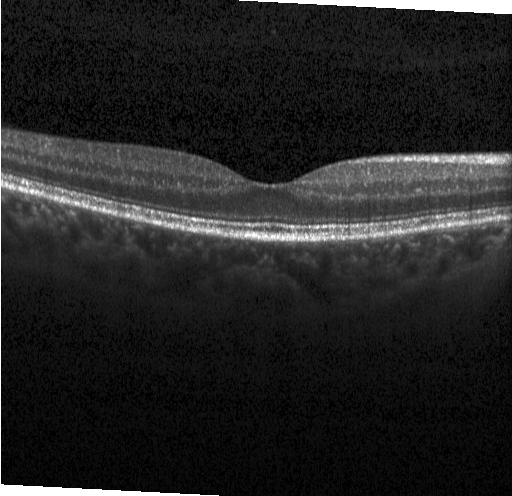 Spectral-domain optical coherence tomography · OCT line scan — Assessment: no evidence of choroidal neovascularization, diabetic macular edema, or drusen.